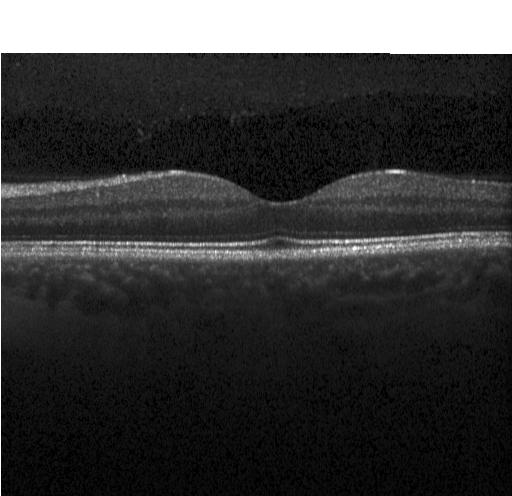 Heidelberg Spectralis; spectral-domain OCT; optical coherence tomography B-scan
Finding: no choroidal neovascularization, diabetic macular edema, or drusen.